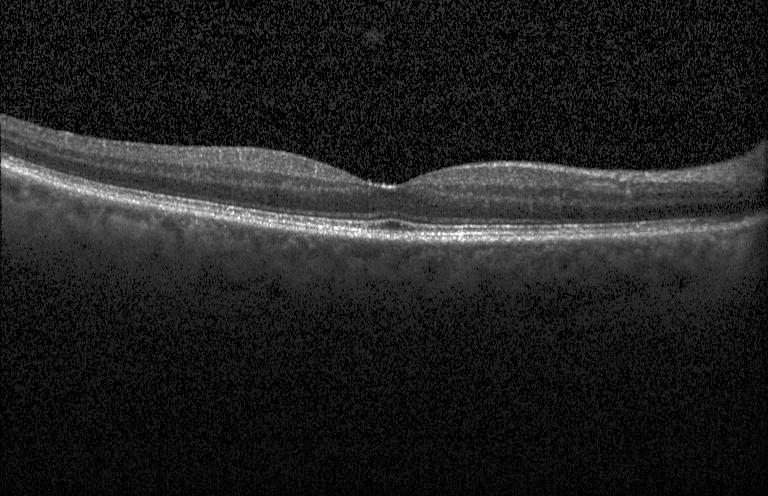 This B-scan demonstrates neither CNV, DME, nor drusen.